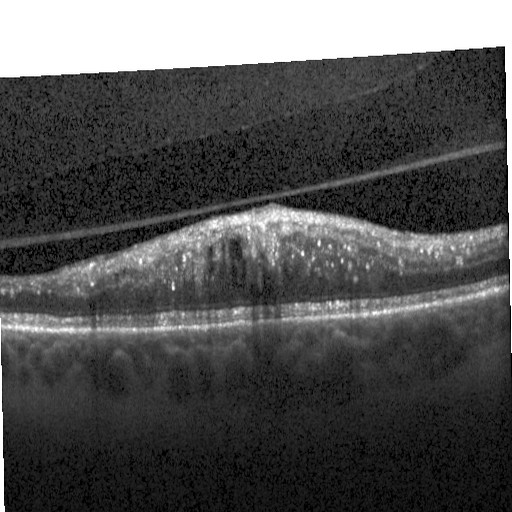 Optical coherence tomography B-scan, SD-OCT
Diabetic macular edema.